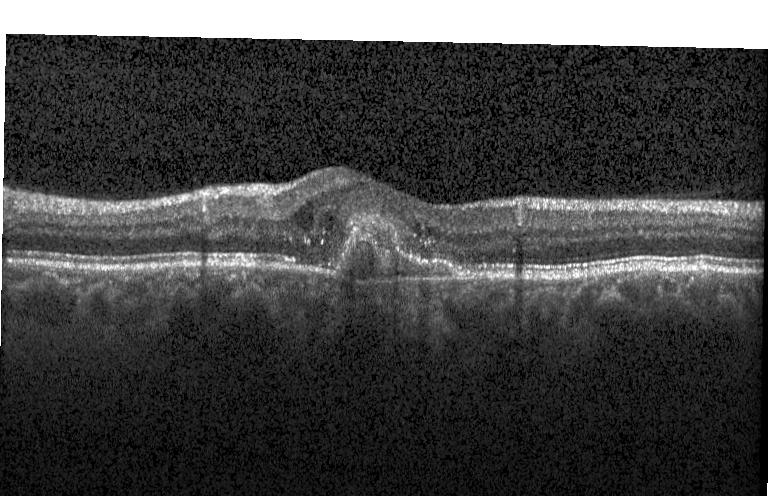
Impression: CNV.